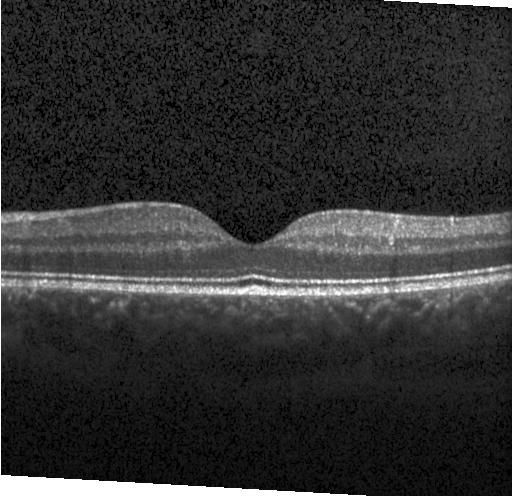

Spectral-domain OCT · centered on the fovea · acquired on a Heidelberg Spectralis · OCT B-scan.
The scan shows no choroidal neovascularization, no diabetic macular edema, and no drusen.